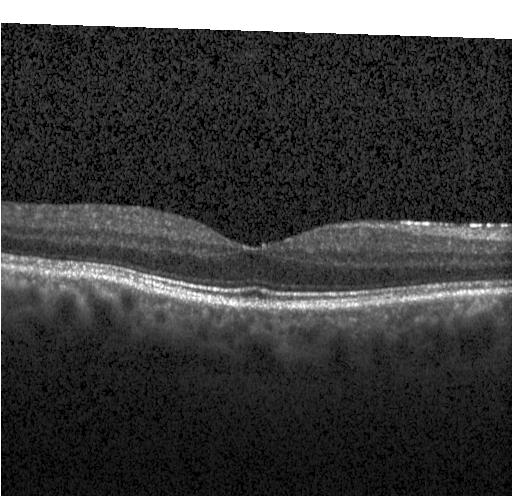 OCT B-scan.
Diagnosis: no choroidal neovascularization, no diabetic macular edema, and no drusen.